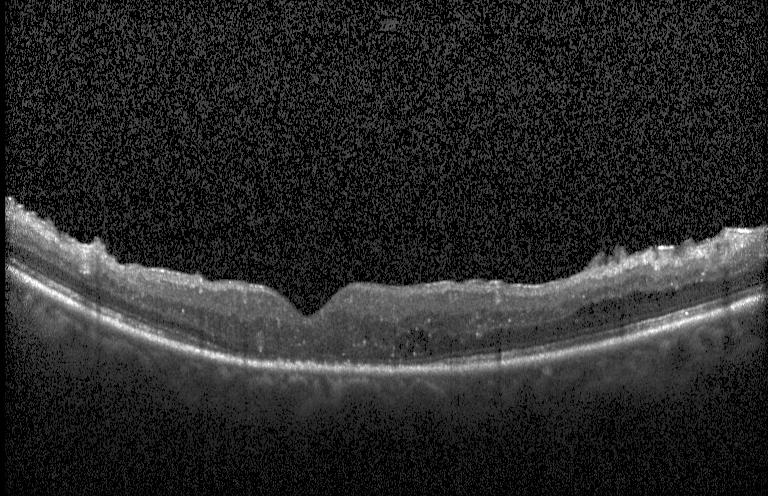
Impression: DME.